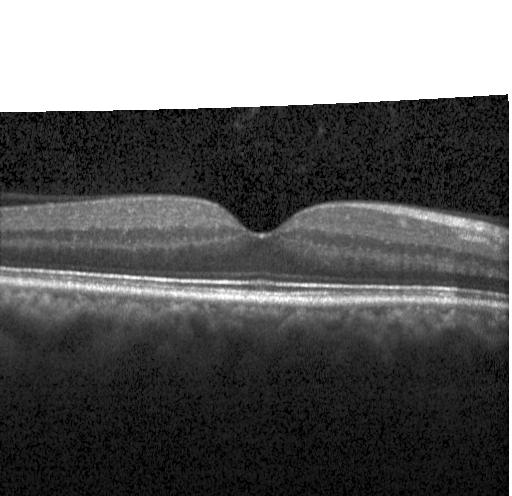

Spectral-domain optical coherence tomography, retinal OCT cross-section.
Dx: no choroidal neovascularization, diabetic macular edema, or drusen.